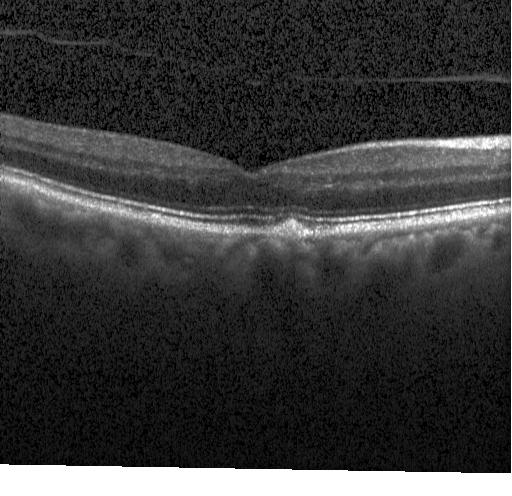

OCT scan showing drusen.